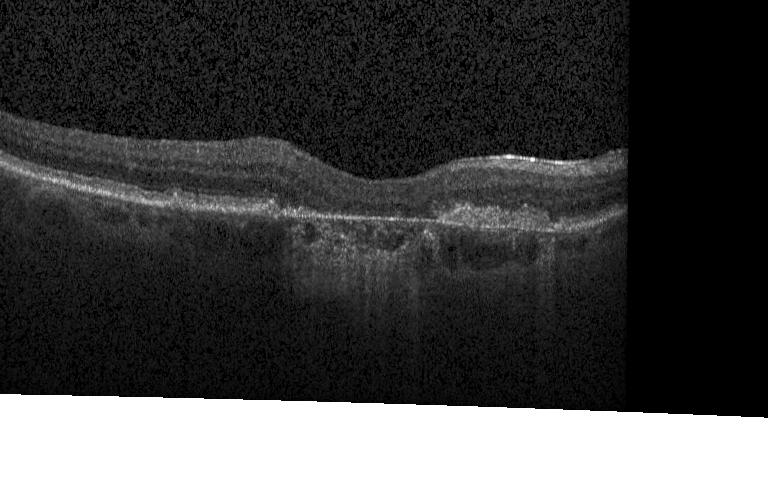
Spectral-domain optical coherence tomography · OCT line scan.
CNV.